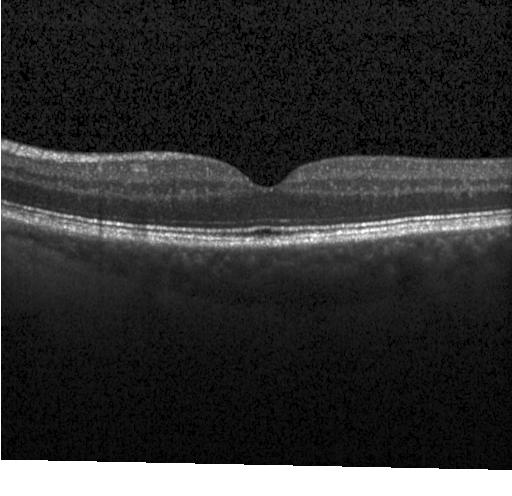 Retinal OCT cross-section; spectral-domain optical coherence tomography.
No CNV, DME, or drusen.